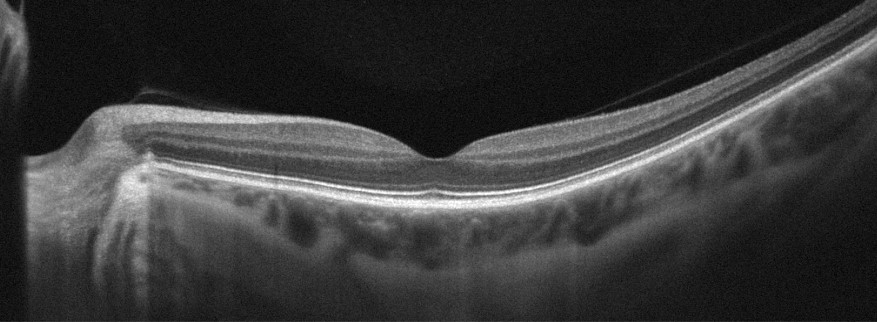

OCT line scan, Optovue Avanti RTVue XR — Finding: absence of AMD, DME, ERM, RAO, RVO, and vitreomacular interface disease.